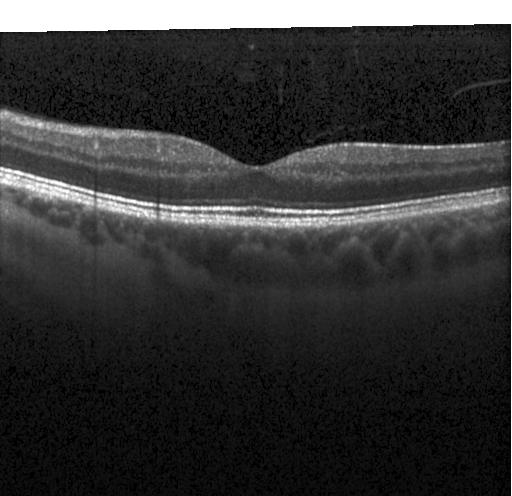
Assessment: no choroidal neovascularization, no diabetic macular edema, and no drusen.